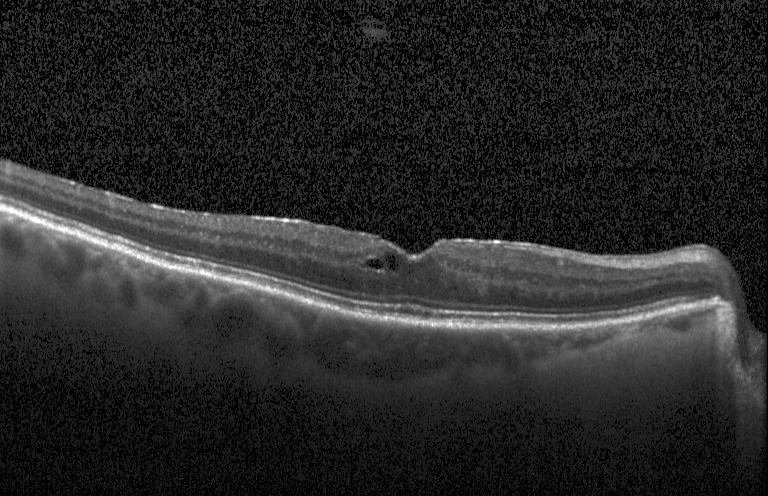
DME.